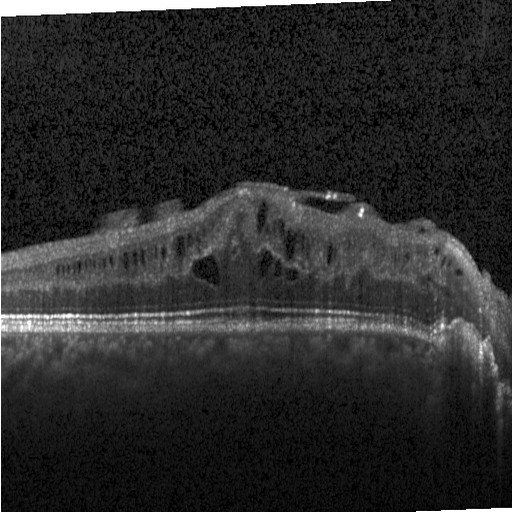

Finding: diabetic macular edema (DME).